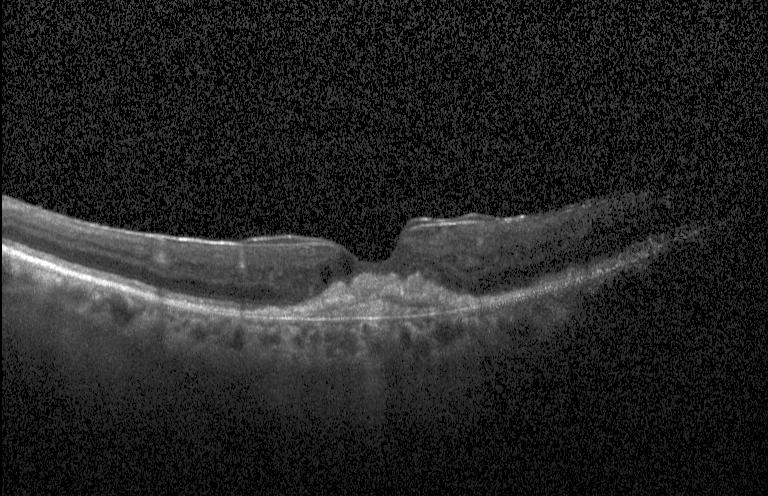

Acquired on a Heidelberg Spectralis; spectral-domain OCT; optical coherence tomography scan. Macular OCT: a choroidal neovascular membrane.